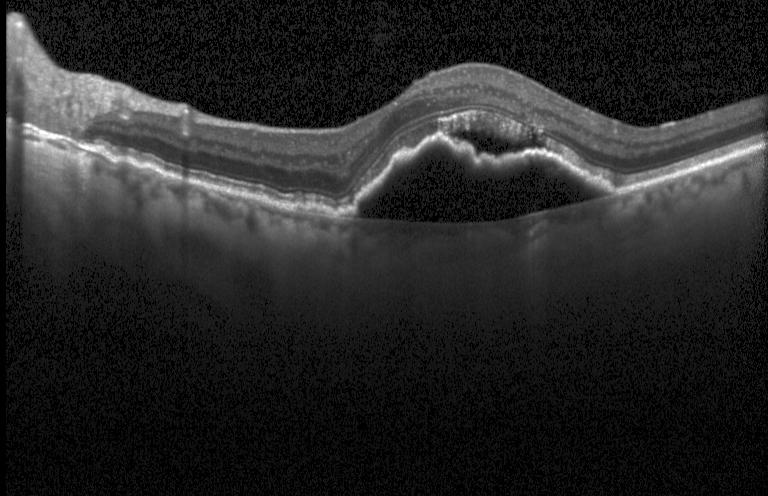
Retinal OCT B-scan, Heidelberg Spectralis OCT system. Macular OCT: a choroidal neovascular membrane.